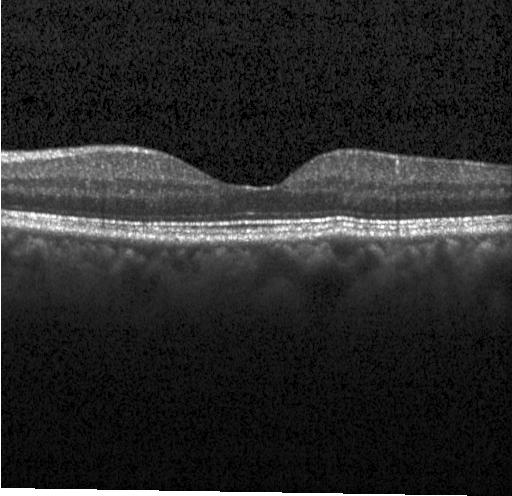
Retinal OCT B-scan.
Finding: neither CNV, DME, nor drusen.